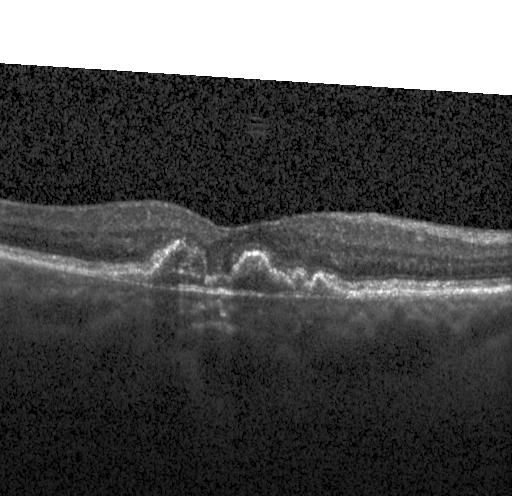
Retinal OCT B-scan, acquired on a Heidelberg Spectralis, spectral-domain OCT
Diagnosis: choroidal neovascularization (CNV).